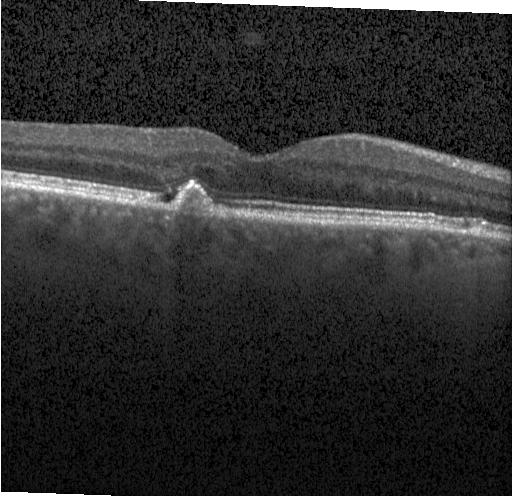

Choroidal neovascularization.